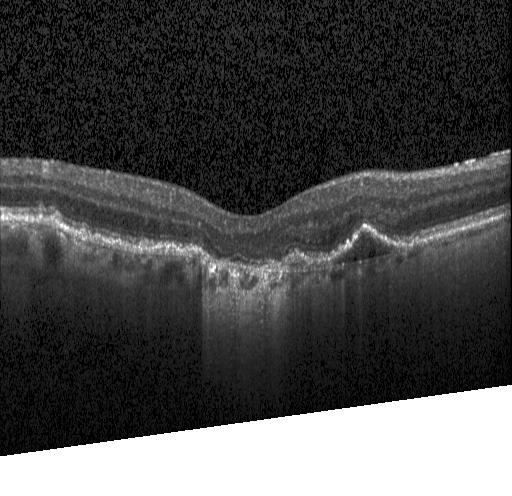

Retinal OCT cross-section, spectral-domain optical coherence tomography, Heidelberg Spectralis OCT system — Diagnosis: choroidal neovascularization (CNV).